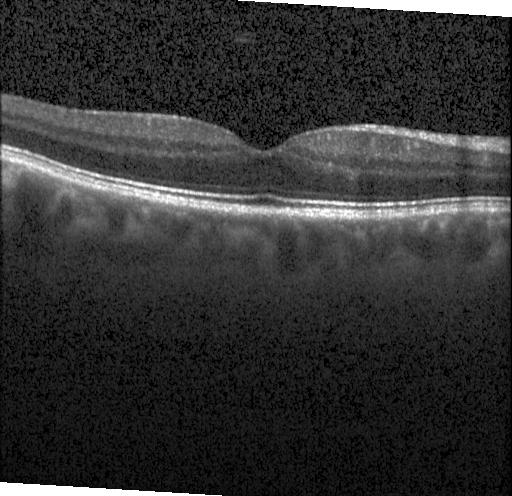 OCT scan showing no evidence of CNV, DME, or drusen.